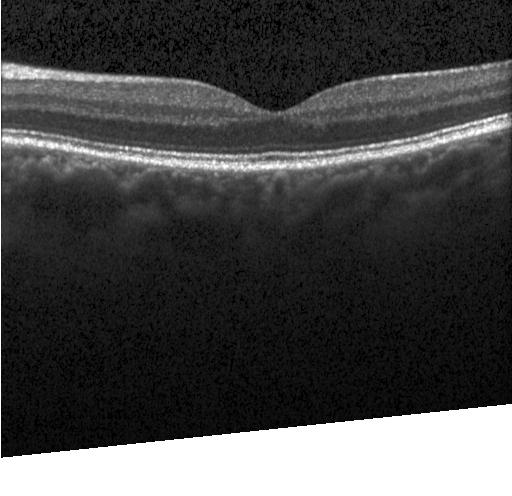
Spectral-domain optical coherence tomography · Heidelberg Spectralis · fovea-centered · retinal OCT cross-section. Macular OCT: no choroidal neovascularization, diabetic macular edema, or drusen.